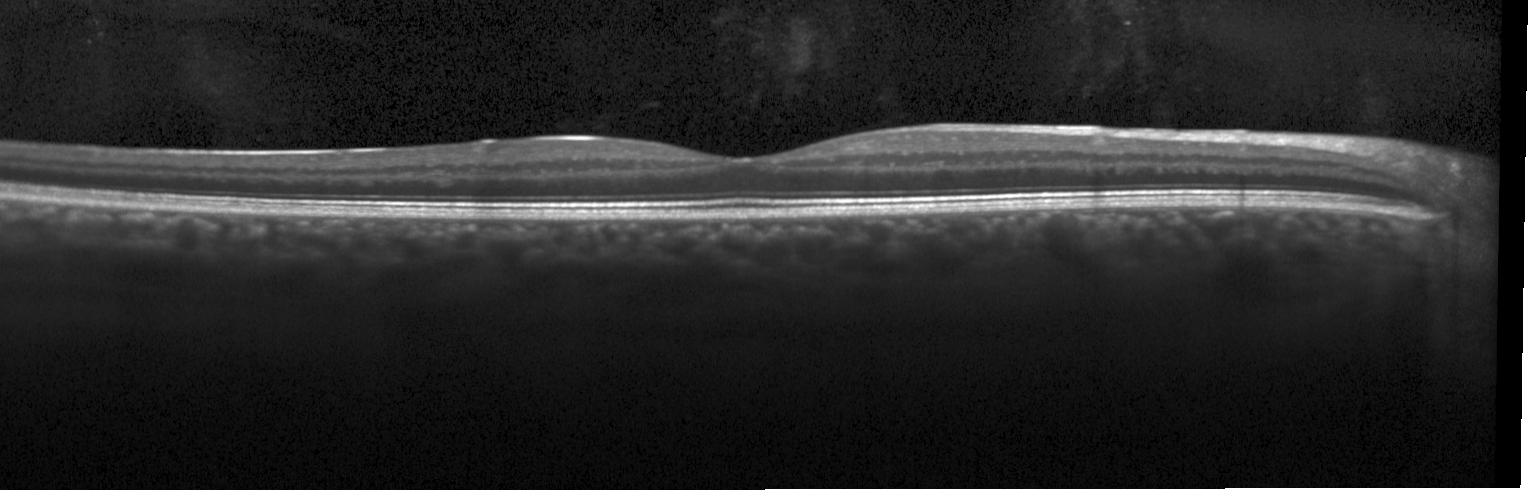 Optical coherence tomography B-scan — OCT finding: no evidence of CNV, DME, or drusen.